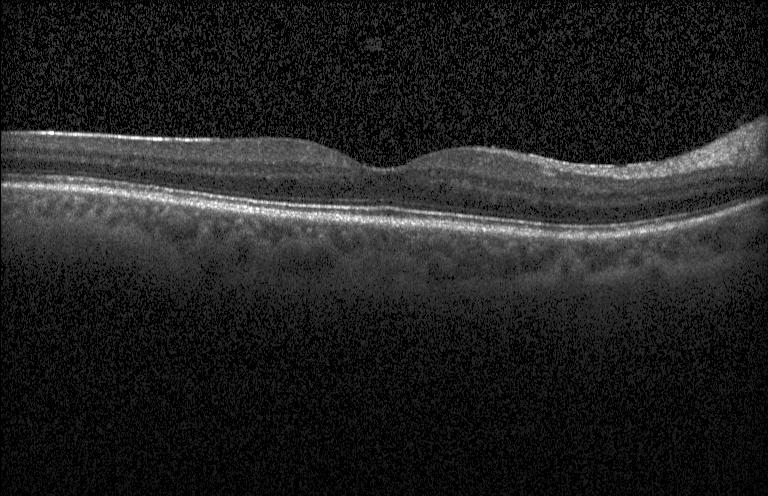
Retinal OCT B-scan.
Impression: neither choroidal neovascularization, diabetic macular edema, nor drusen.